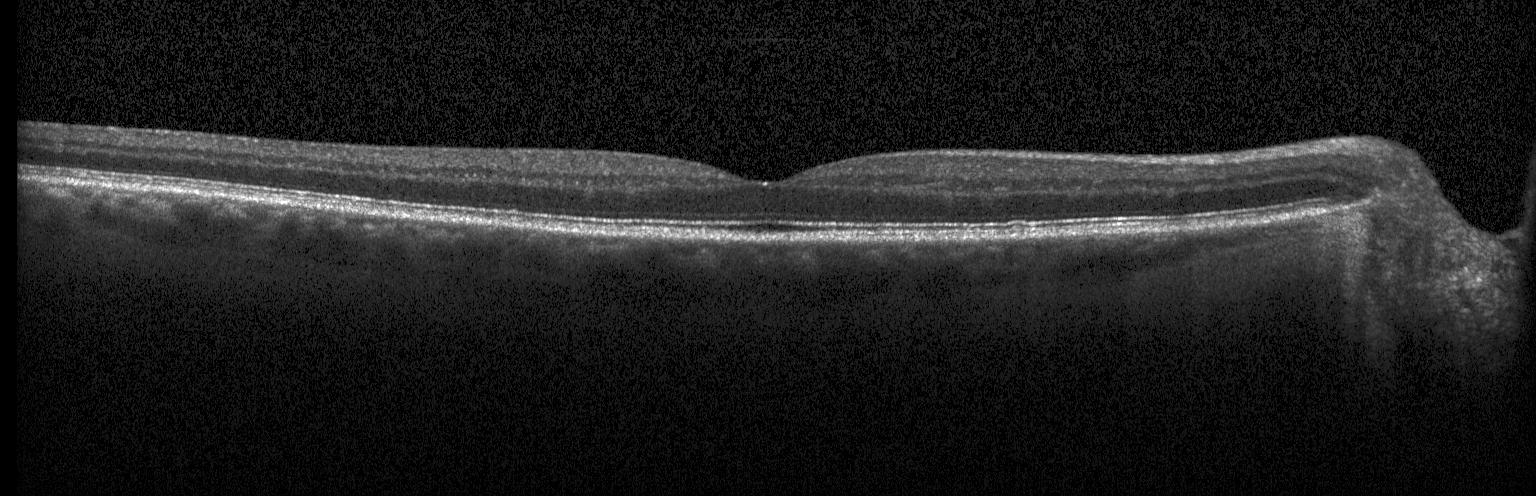
OCT B-scan showing no choroidal neovascularization, no diabetic macular edema, and no drusen.